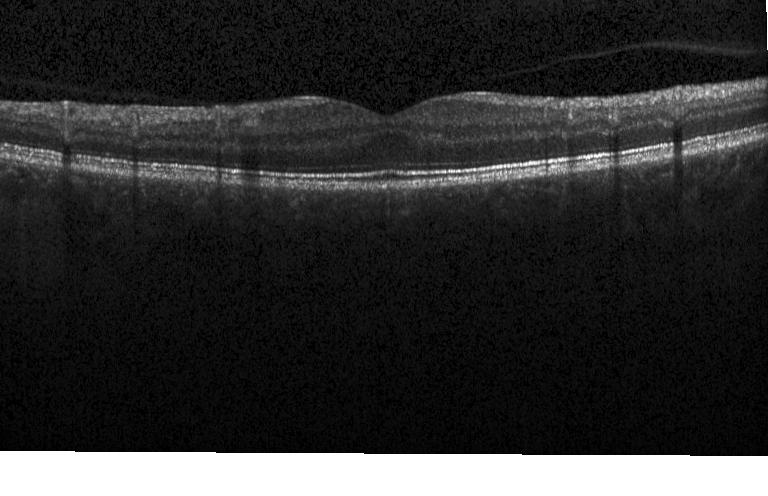 The scan shows no evidence of choroidal neovascularization, diabetic macular edema, or drusen.